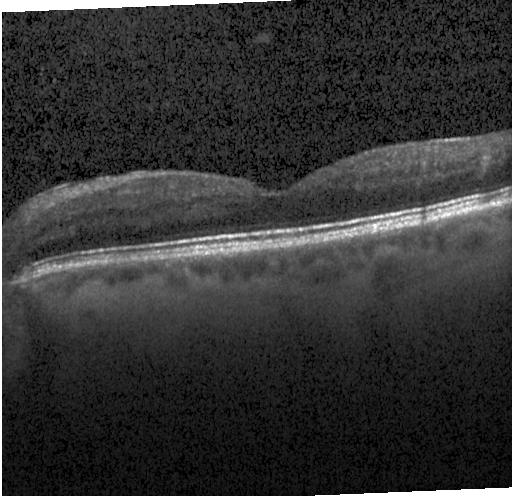

Acquired on a Heidelberg Spectralis, spectral-domain OCT, retinal OCT B-scan
Diagnosis: no choroidal neovascularization, no diabetic macular edema, and no drusen.